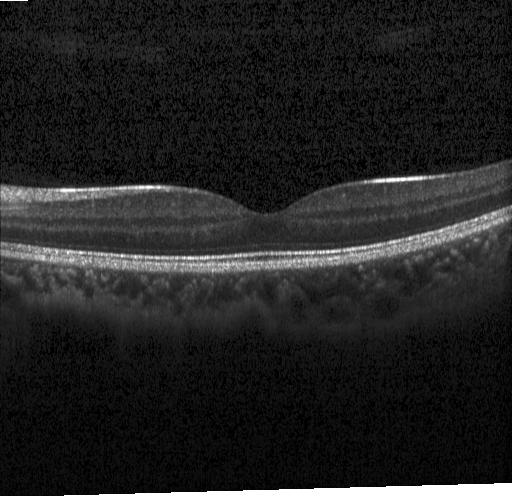
SD-OCT · OCT line scan · Heidelberg Spectralis
Macular OCT: no choroidal neovascularization, diabetic macular edema, or drusen.